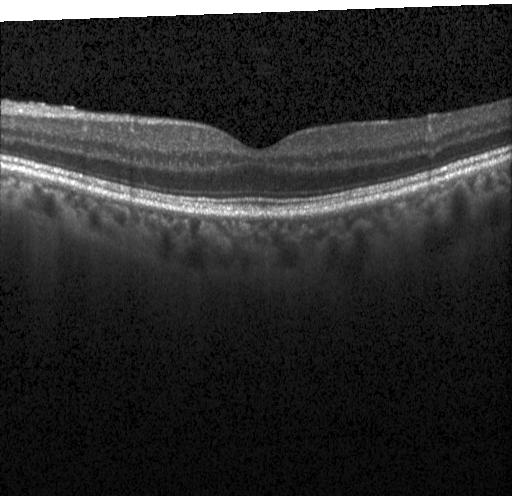

Macular OCT: no choroidal neovascularization, diabetic macular edema, or drusen.